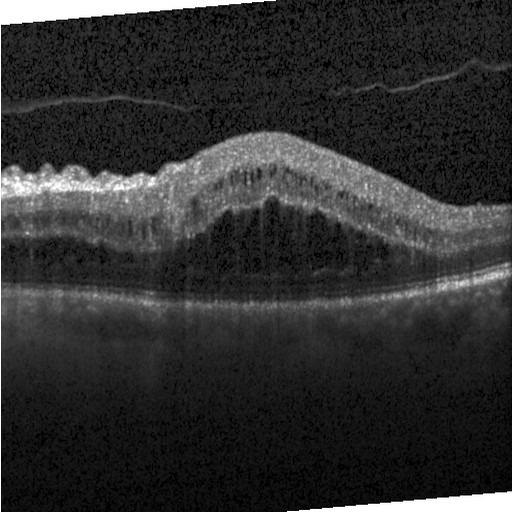 Heidelberg Spectralis OCT system. Horizontal scan through the fovea. Optical coherence tomography scan. Assessment: diabetic macular edema (DME).